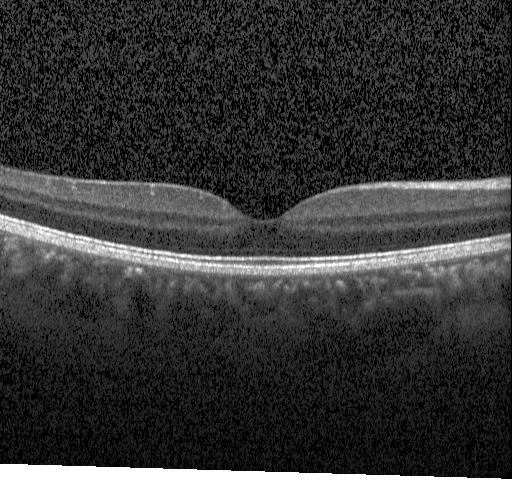
No evidence of choroidal neovascularization, diabetic macular edema, or drusen.